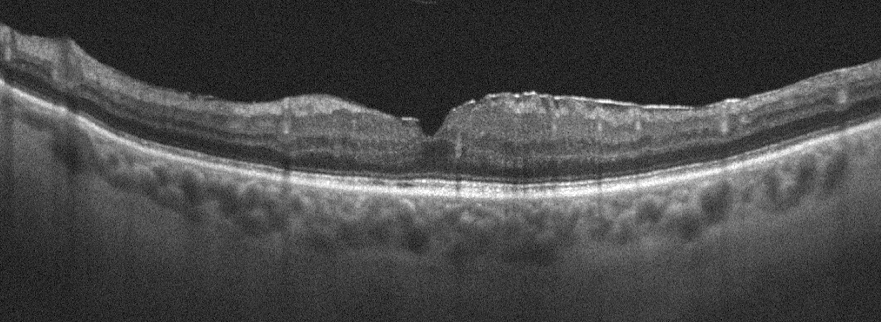

Retinal OCT cross-section. Assessment: epiretinal membrane (ERM).